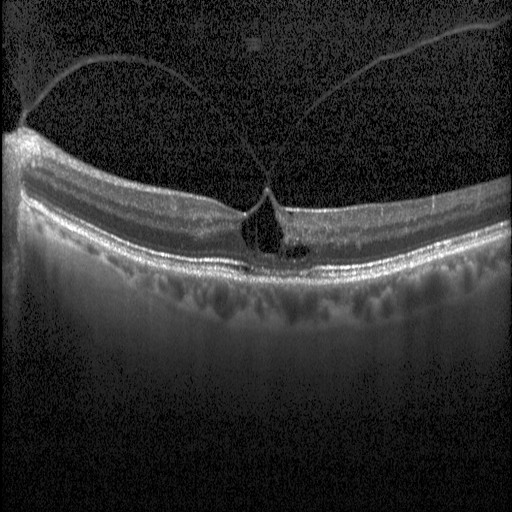

Optical coherence tomography B-scan. Finding: diabetic macular edema.